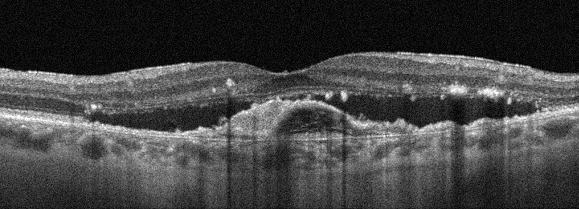
OCT line scan · OS — Macular OCT: age-related macular degeneration (AMD).